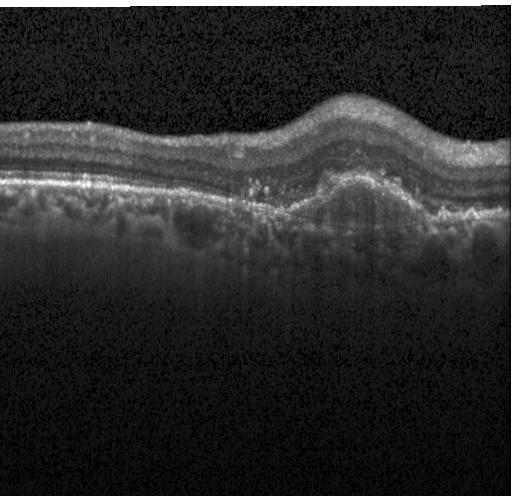

Retinal OCT cross-section; Heidelberg Spectralis OCT system; SD-OCT; through the macula.
Diagnosis: choroidal neovascularization.